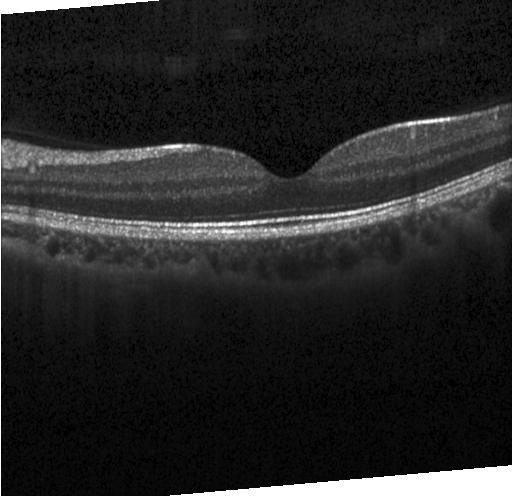 Centered on the fovea; OCT line scan; spectral-domain OCT.
No evidence of choroidal neovascularization, diabetic macular edema, or drusen.